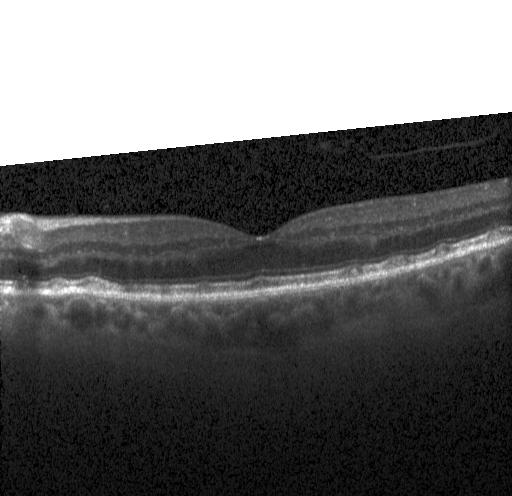
Heidelberg Spectralis OCT system. Retinal OCT cross-section. Spectral-domain OCT
Impression: sub-RPE drusenoid deposits.